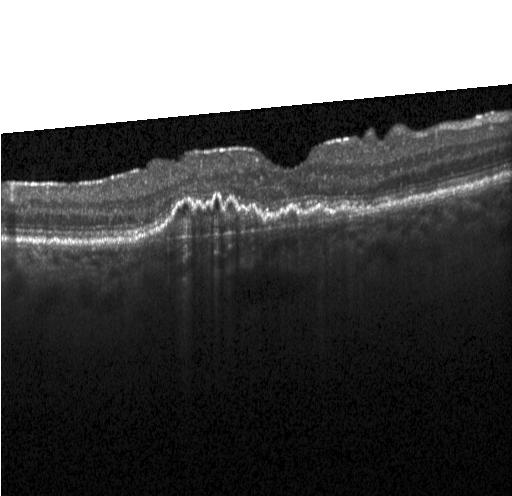
Finding: a choroidal neovascular membrane.